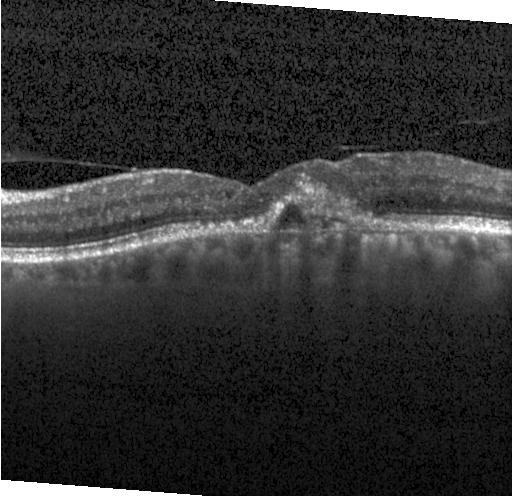 OCT scan showing a choroidal neovascular membrane.